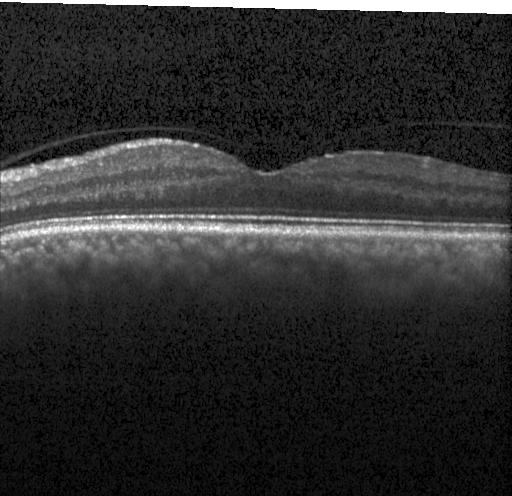

OCT line scan — Finding: no choroidal neovascularization, no diabetic macular edema, and no drusen.